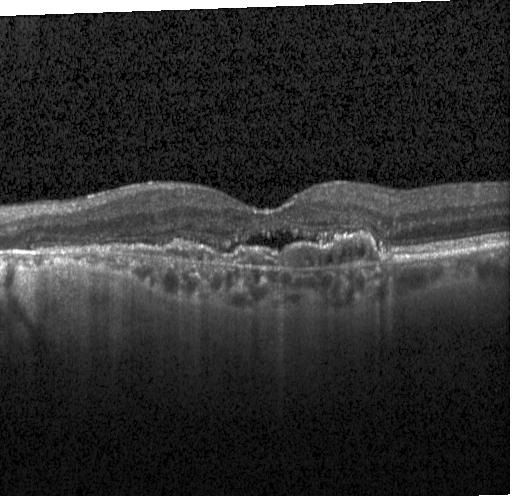

OCT line scan — Impression: a choroidal neovascular membrane.